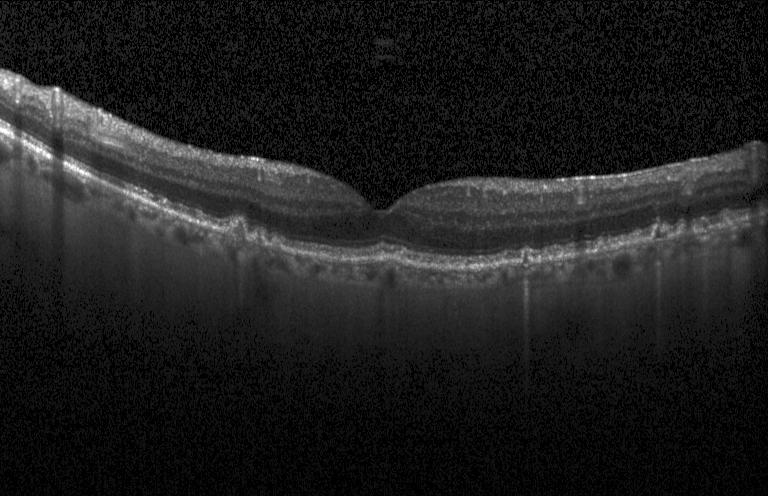
Drusen.